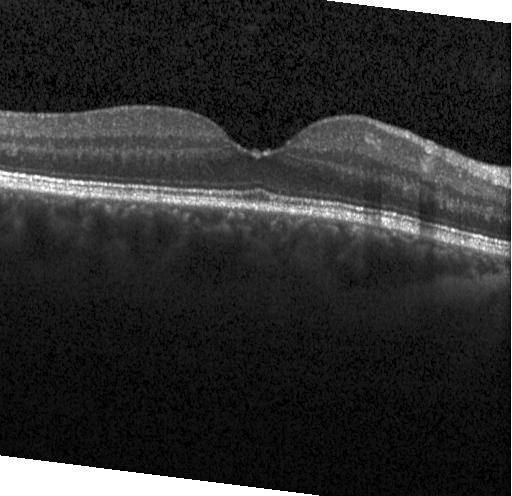 Spectral-domain OCT B-scan: no evidence of CNV, DME, or drusen.